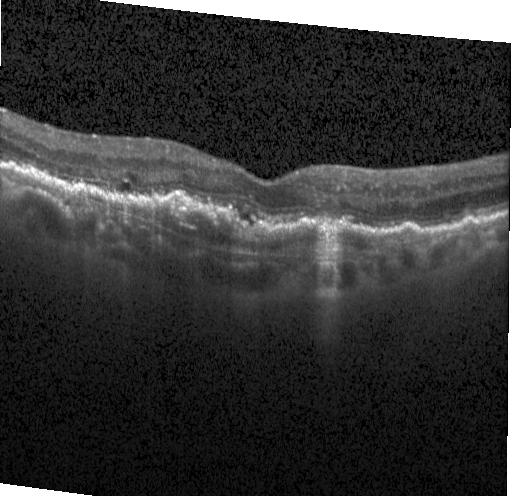

Spectral-domain optical coherence tomography · retinal OCT cross-section · Heidelberg Spectralis
Impression: choroidal neovascularization.